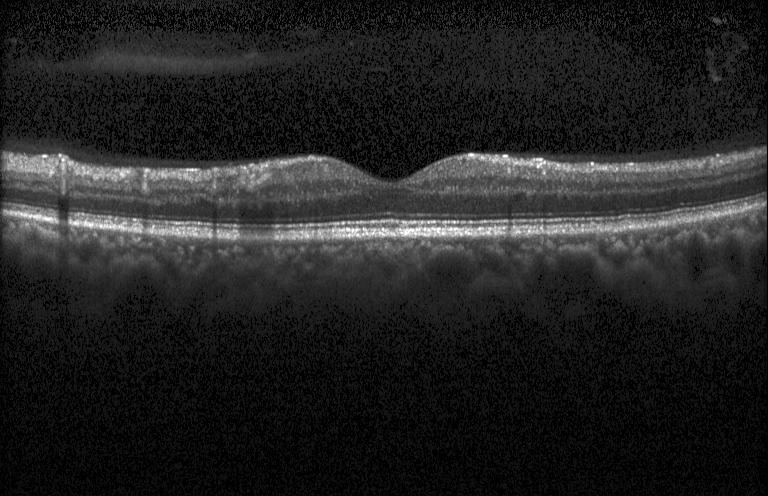

OCT line scan, Heidelberg Spectralis OCT system, spectral-domain OCT — Impression: neither choroidal neovascularization, diabetic macular edema, nor drusen.